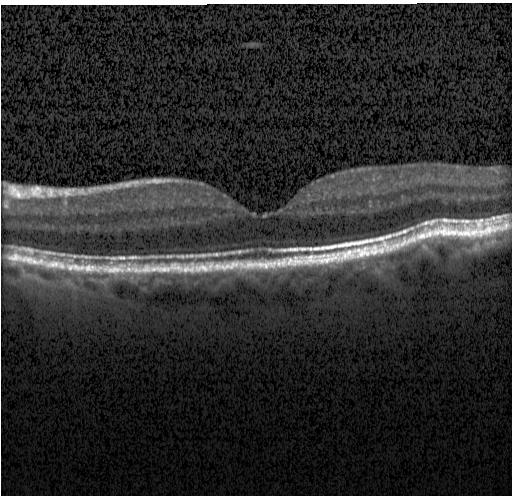
Impression: no choroidal neovascularization, diabetic macular edema, or drusen.